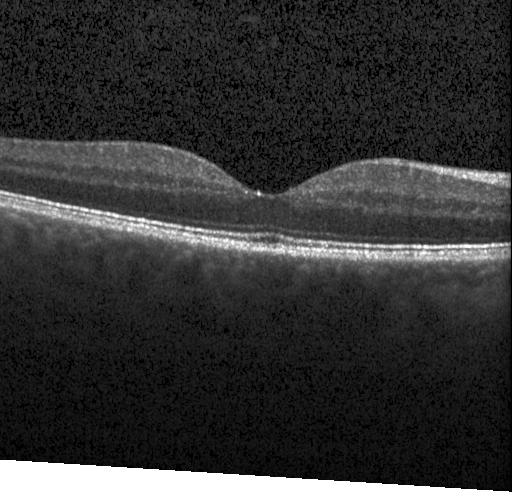

Optical coherence tomography scan.
Assessment: no choroidal neovascularization, diabetic macular edema, or drusen.